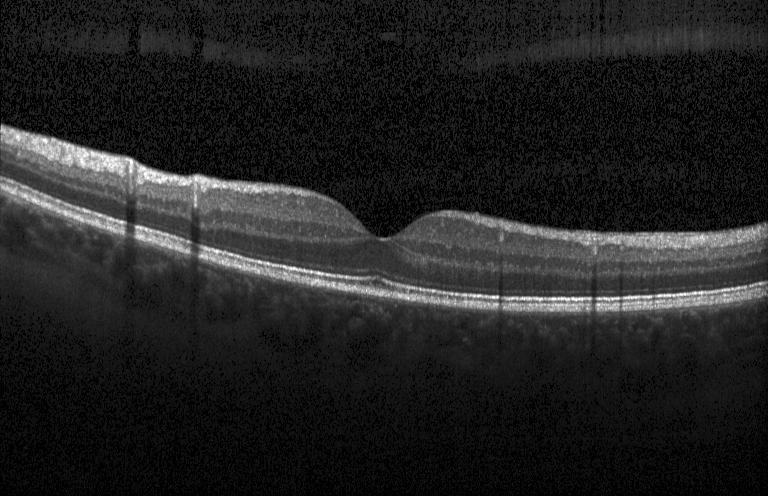
Optical coherence tomography scan
Impression: no choroidal neovascularization, no diabetic macular edema, and no drusen.